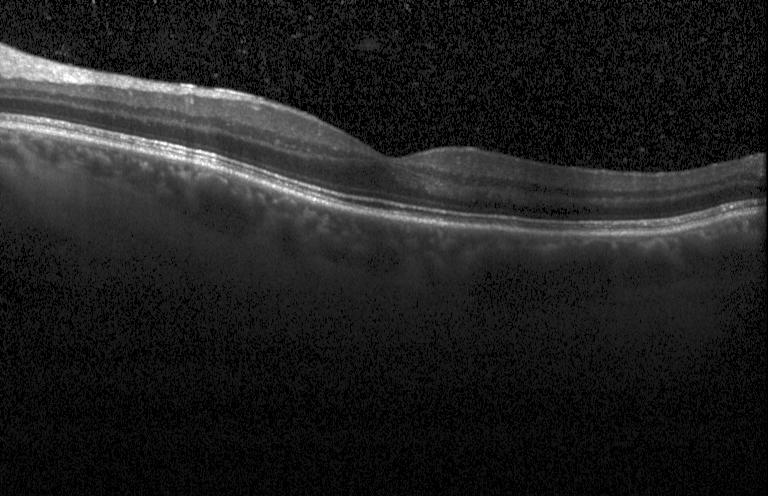
OCT B-scan · Heidelberg Spectralis OCT system · SD-OCT — Assessment: no evidence of choroidal neovascularization, diabetic macular edema, or drusen.